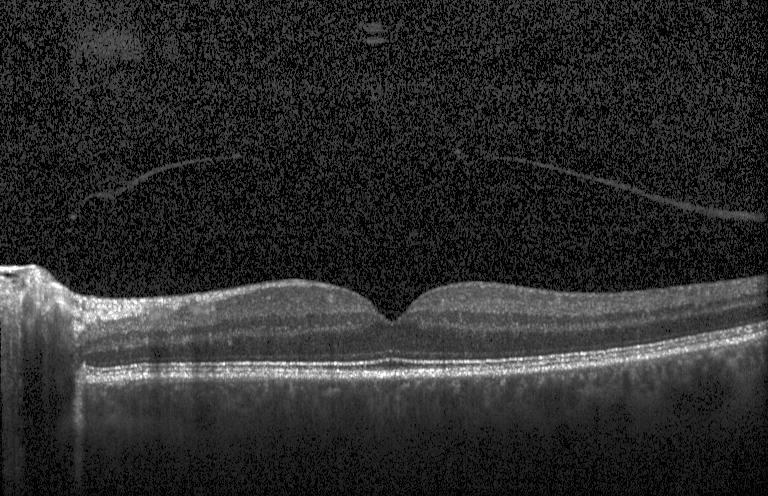

Retinal OCT cross-section. Finding: no evidence of CNV, DME, or drusen.